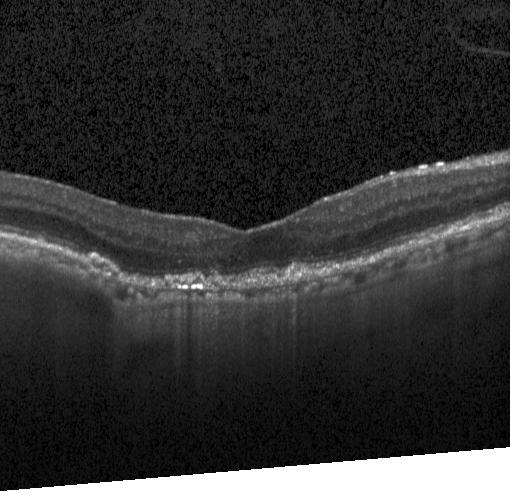
Optical coherence tomography scan. Macular OCT: choroidal neovascularization.